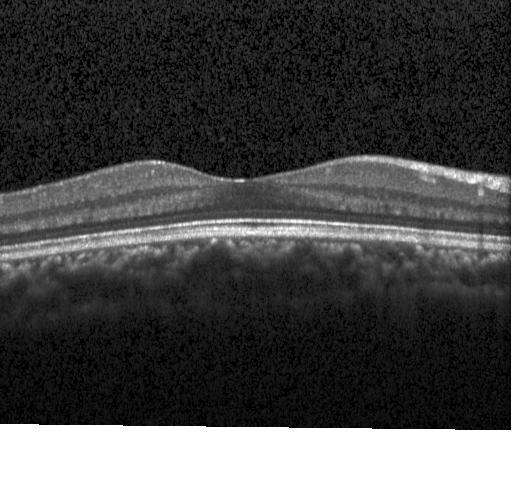
Retinal OCT cross-section — OCT finding: no evidence of CNV, DME, or drusen.